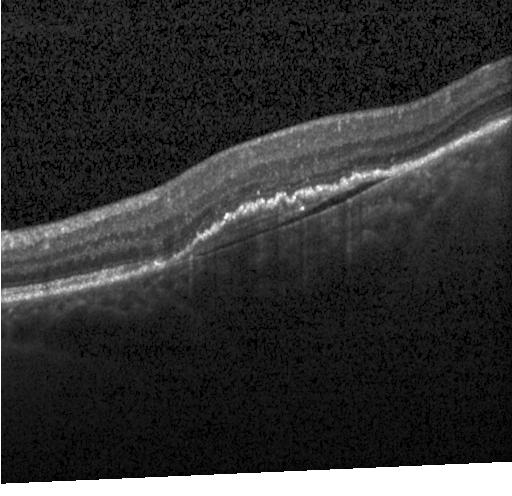 Spectral-domain optical coherence tomography, optical coherence tomography scan, Heidelberg Spectralis OCT system.
Diagnosis: CNV.